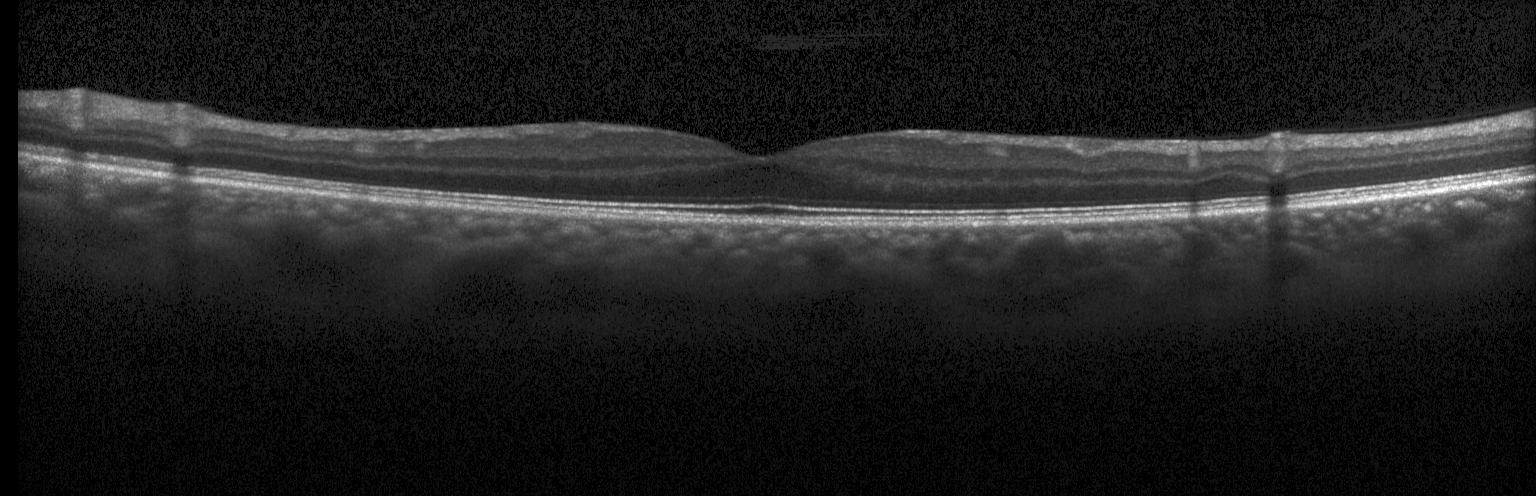
Impression: no choroidal neovascularization, diabetic macular edema, or drusen.